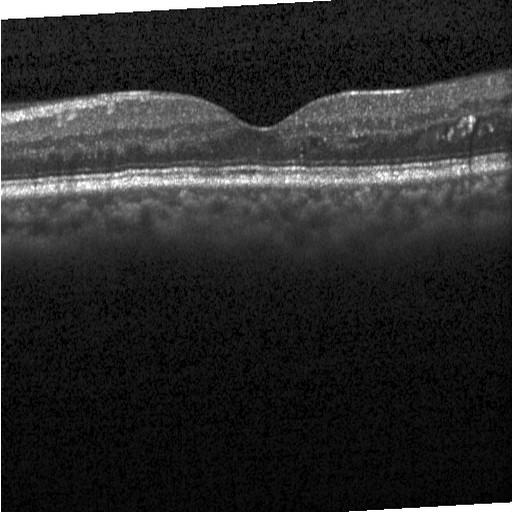 Optical coherence tomography scan · instrument: Heidelberg Spectralis
Assessment: diabetic macular edema (DME).